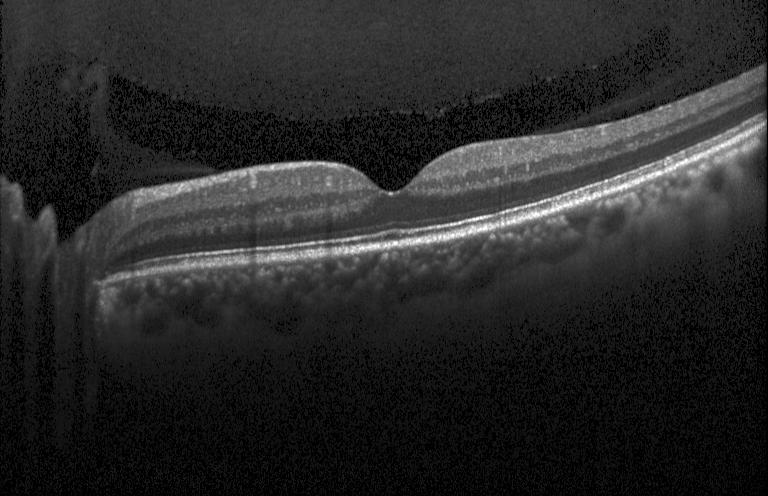 Macular OCT: no evidence of choroidal neovascularization, diabetic macular edema, or drusen.